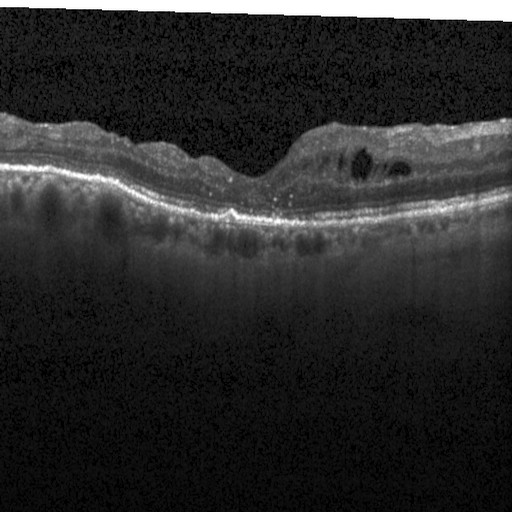
OCT B-scan
Diagnosis: diabetic macular edema (DME).